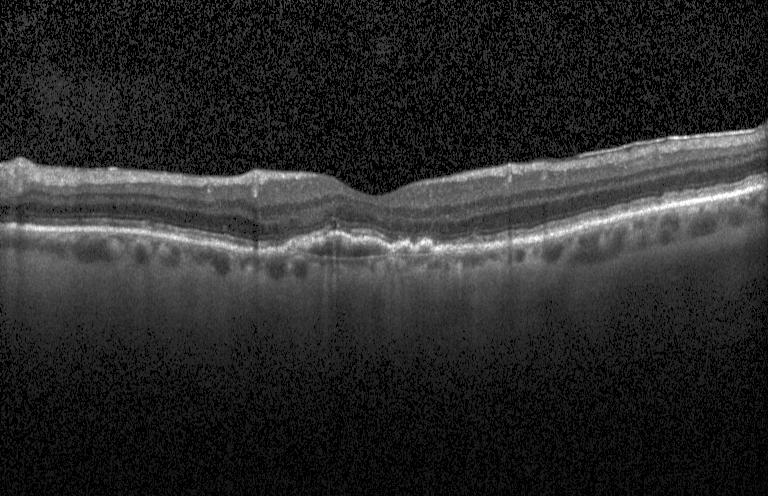
Spectral-domain optical coherence tomography; retinal OCT cross-section — A choroidal neovascular membrane.